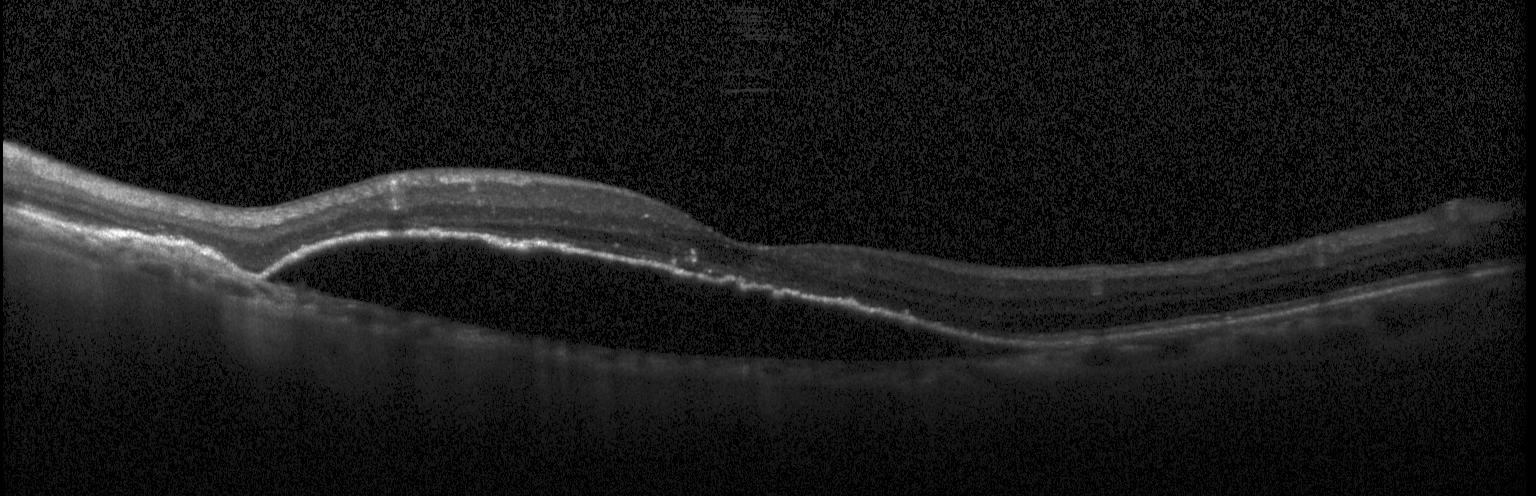 Heidelberg Spectralis. Optical coherence tomography B-scan. Impression: choroidal neovascularization.